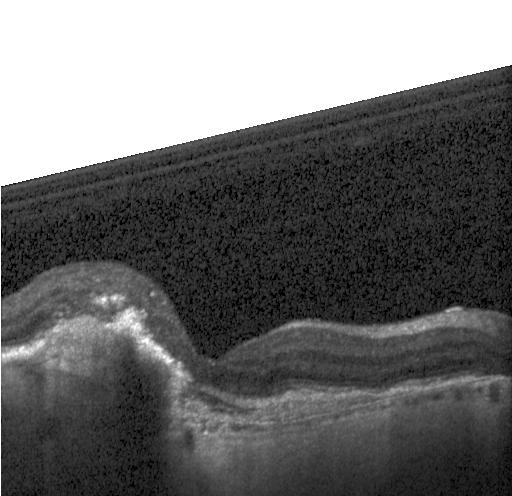
Spectral-domain OCT. OCT line scan. Acquired on a Heidelberg Spectralis. Impression: a choroidal neovascular membrane.